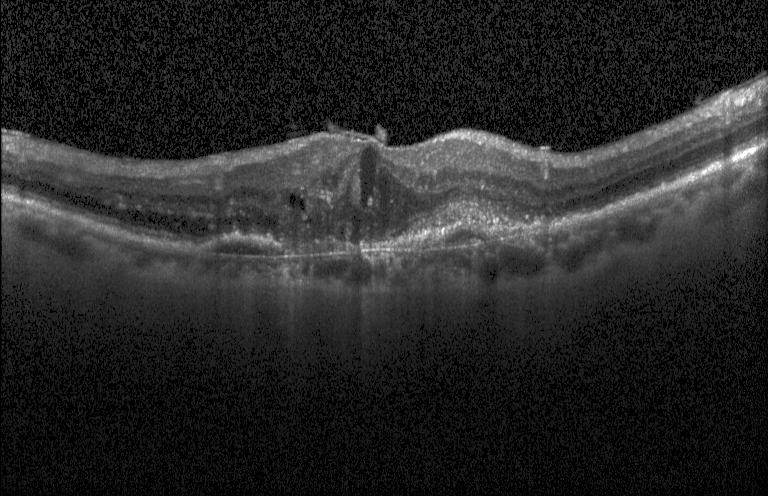

Impression: a choroidal neovascular membrane.